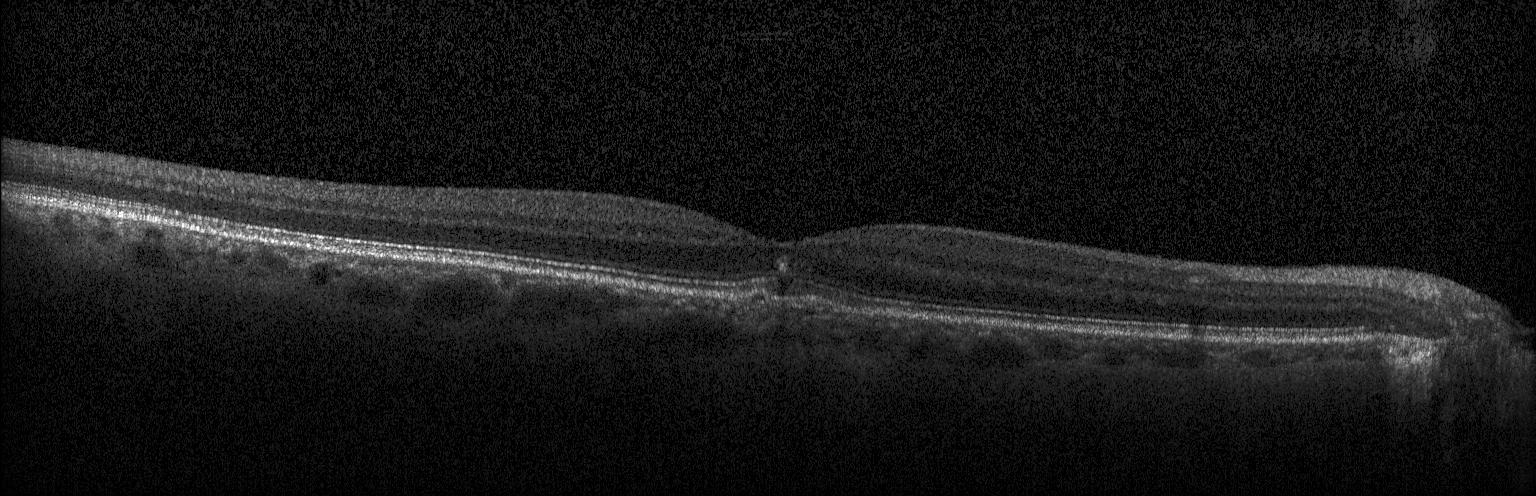 Finding: a choroidal neovascular membrane.